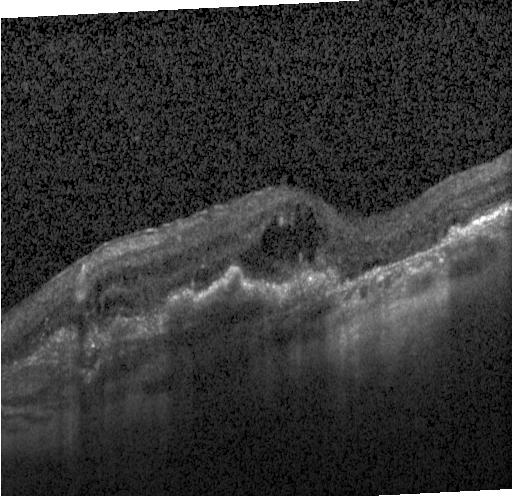 Impression: choroidal neovascularization.